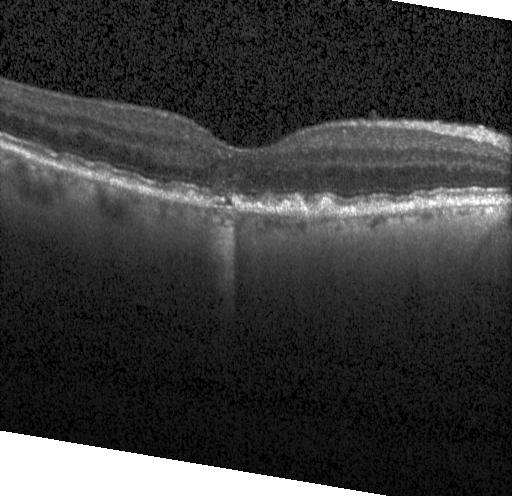

OCT scan showing multiple drusen.